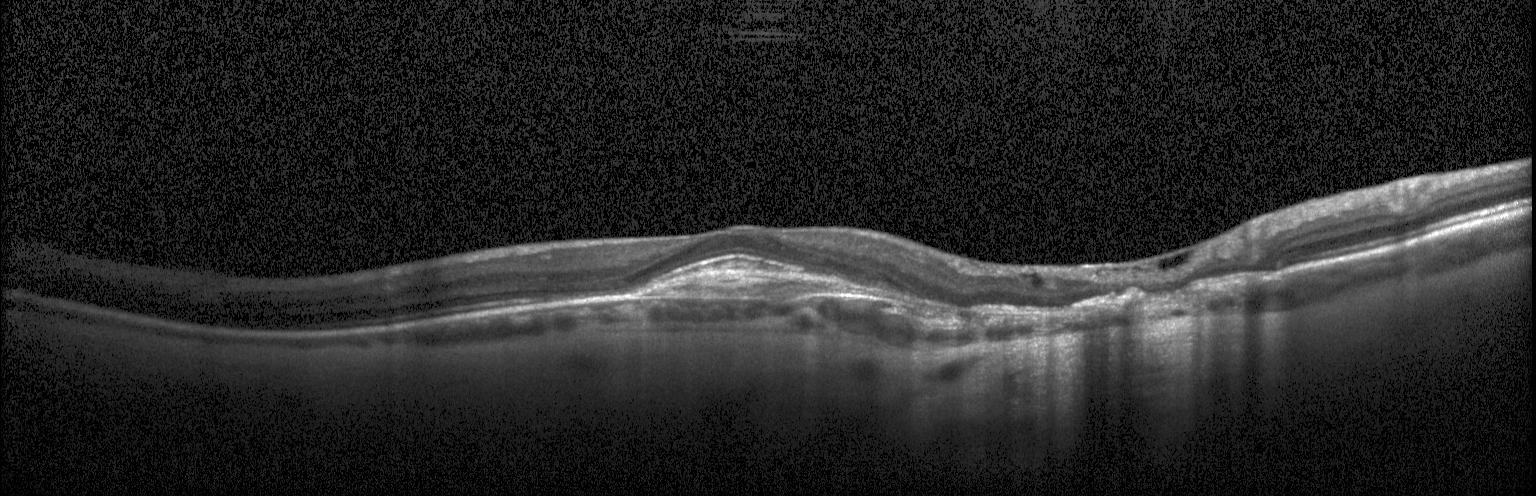
Instrument: Heidelberg Spectralis. OCT B-scan. Centered on the fovea. SD-OCT — Diagnosis: a choroidal neovascular membrane.